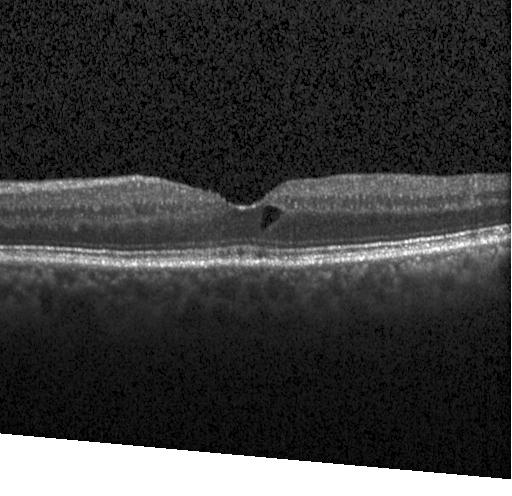
OCT B-scan.
This B-scan demonstrates diabetic macular edema (DME).